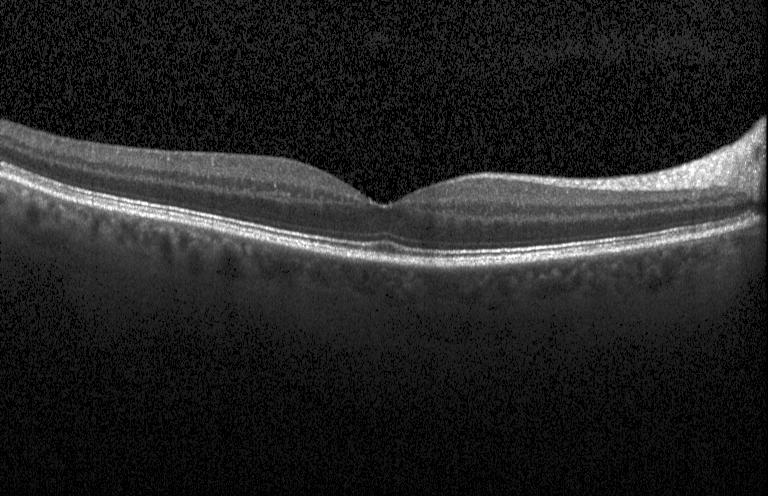
Diagnosis: no choroidal neovascularization, diabetic macular edema, or drusen.